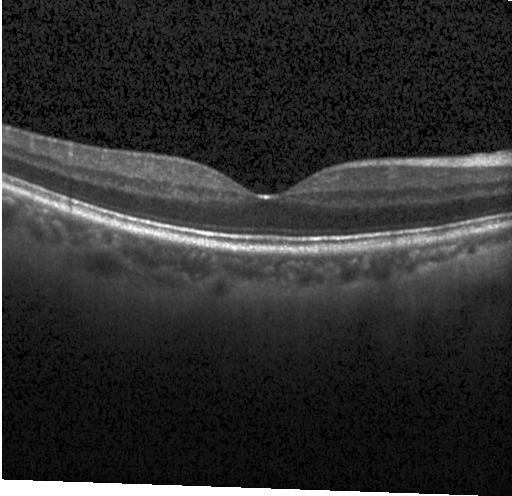
OCT B-scan — Impression: no choroidal neovascularization, diabetic macular edema, or drusen.